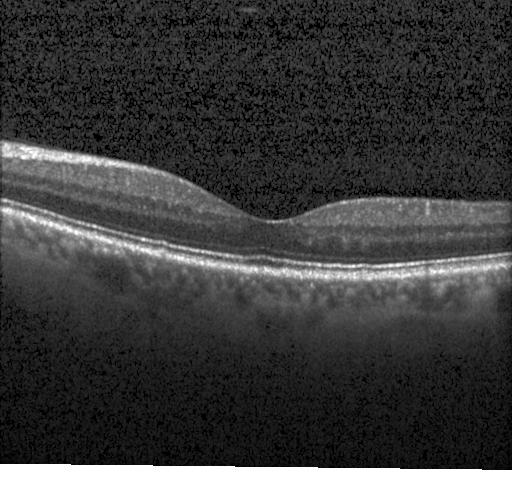 OCT line scan; spectral-domain OCT; instrument: Heidelberg Spectralis; centered on the fovea.
This B-scan demonstrates no evidence of CNV, DME, or drusen.